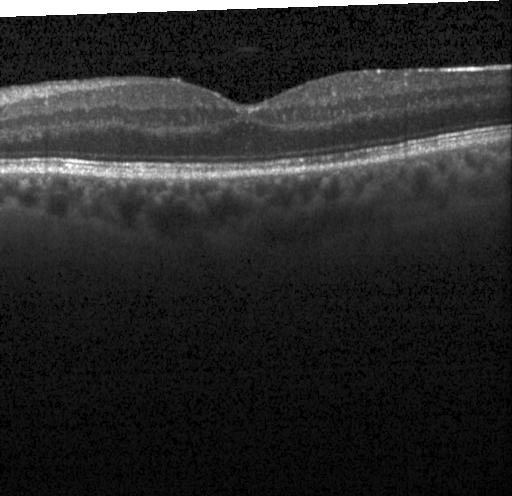

No evidence of CNV, DME, or drusen.